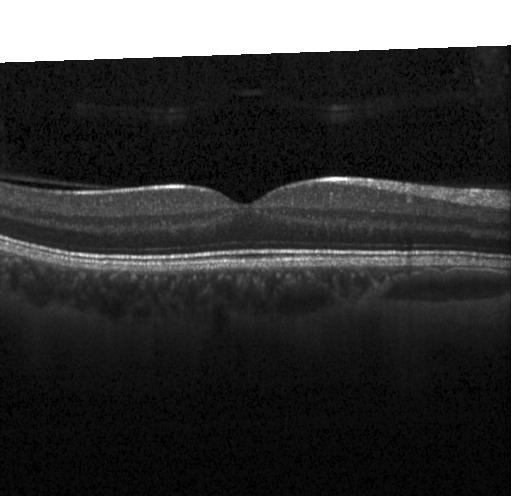
Spectral-domain optical coherence tomography · acquired on a Heidelberg Spectralis · macular scan · optical coherence tomography B-scan. Diagnosis: no choroidal neovascularization, diabetic macular edema, or drusen.